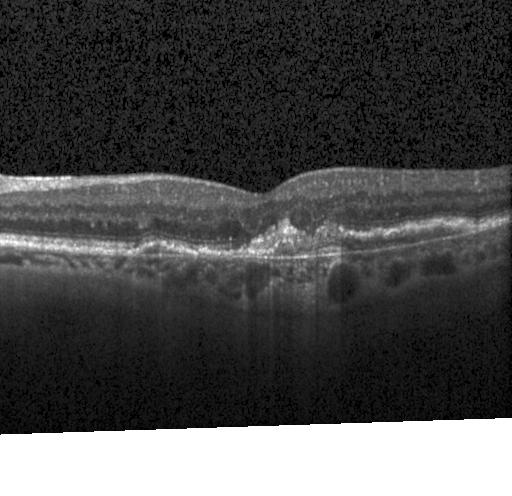
Optical coherence tomography B-scan.
A choroidal neovascular membrane.